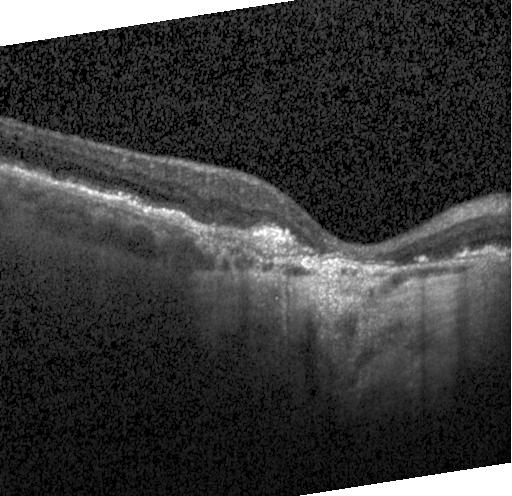 Impression: choroidal neovascularization (CNV).